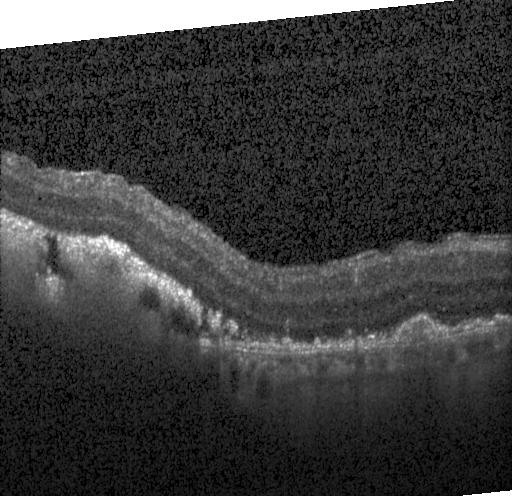
Acquired on a Heidelberg Spectralis, through the macula, retinal OCT cross-section, spectral-domain OCT.
The scan shows choroidal neovascularization (CNV).